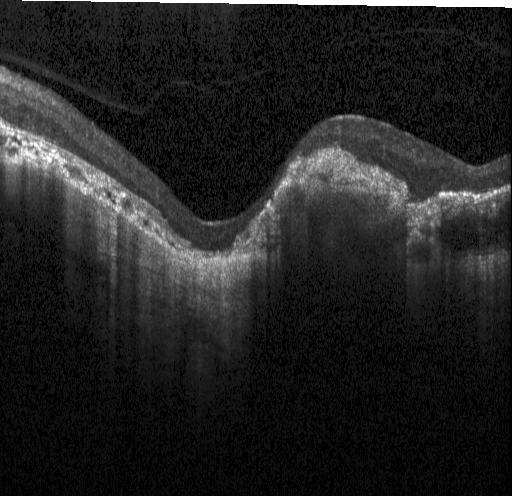

Through the macula · OCT B-scan.
Choroidal neovascularization.